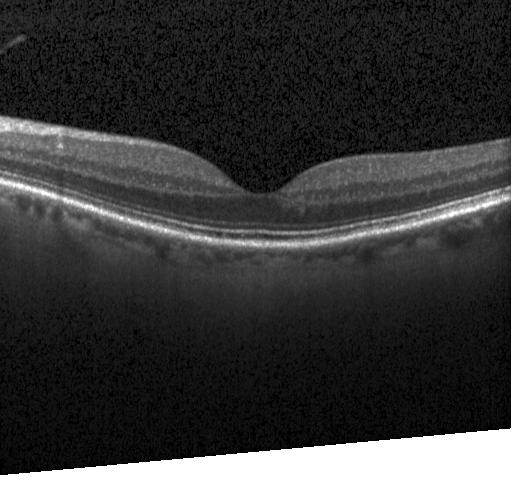 Through the macula; optical coherence tomography scan; SD-OCT; Heidelberg Spectralis. Impression: no evidence of choroidal neovascularization, diabetic macular edema, or drusen.